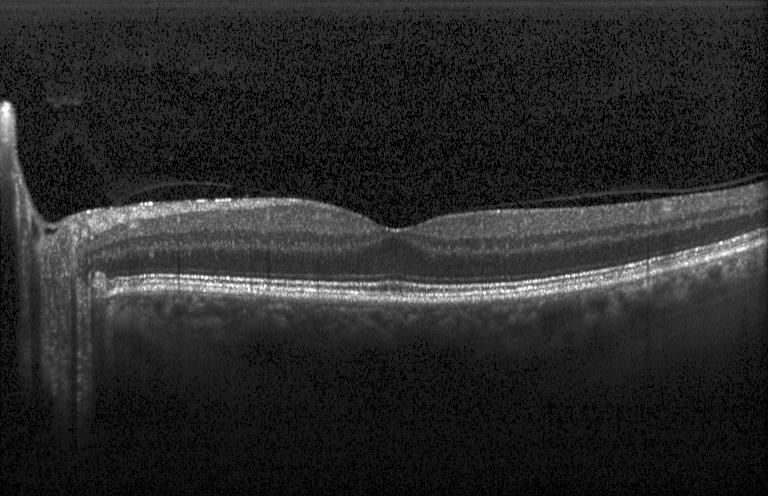

Heidelberg Spectralis; spectral-domain optical coherence tomography; retinal OCT B-scan.
Assessment: neither choroidal neovascularization, diabetic macular edema, nor drusen.